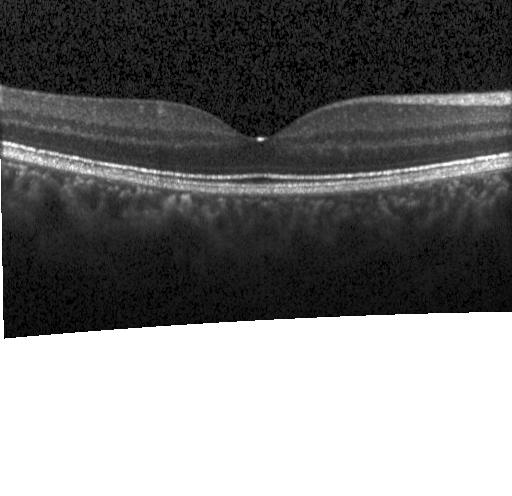

Finding: no CNV, no DME, and no drusen.